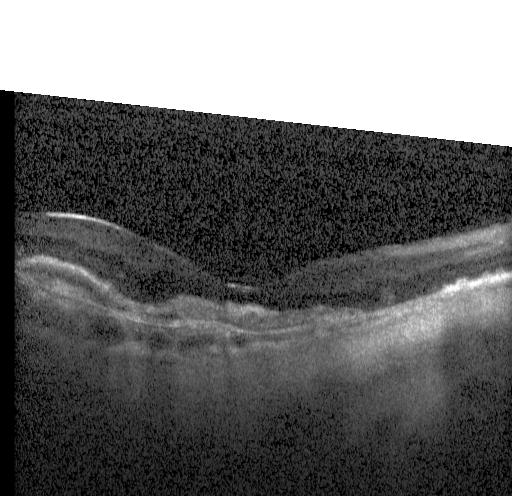

OCT B-scan; acquired on a Heidelberg Spectralis; spectral-domain OCT
This B-scan demonstrates CNV.